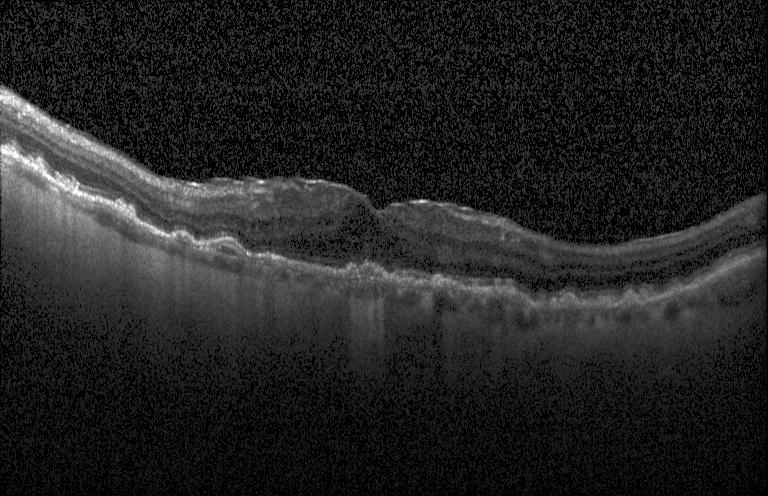 Centered on the fovea. Retinal OCT B-scan. Heidelberg Spectralis OCT system. SD-OCT
Impression: a choroidal neovascular membrane.